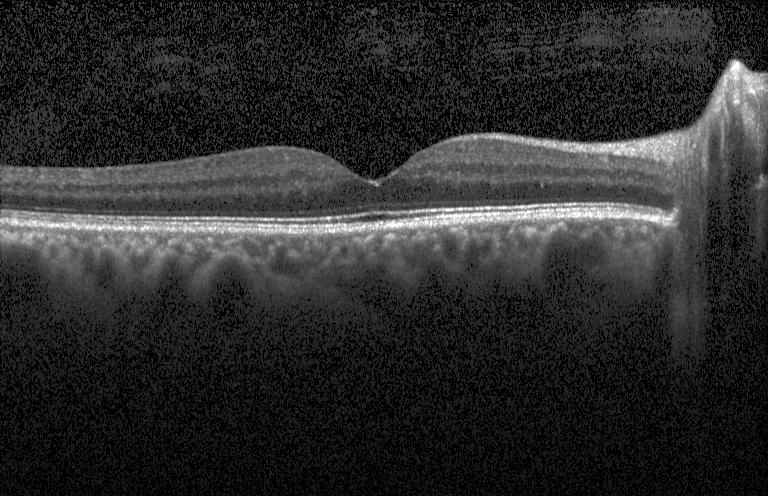 OCT scan showing neither CNV, DME, nor drusen.